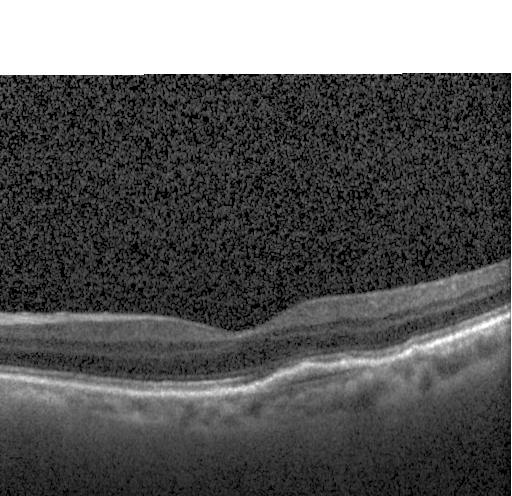
Impression: a choroidal neovascular membrane.